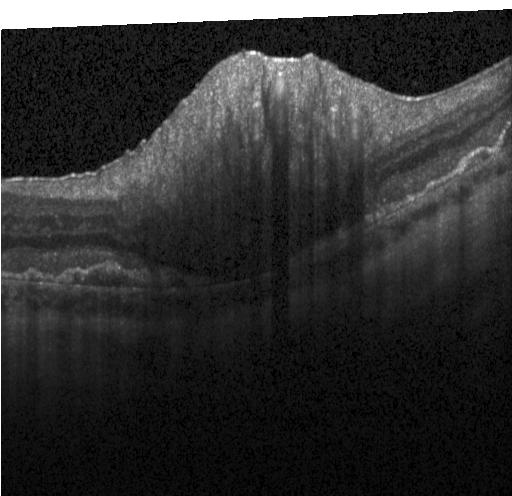

Impression: choroidal neovascularization.